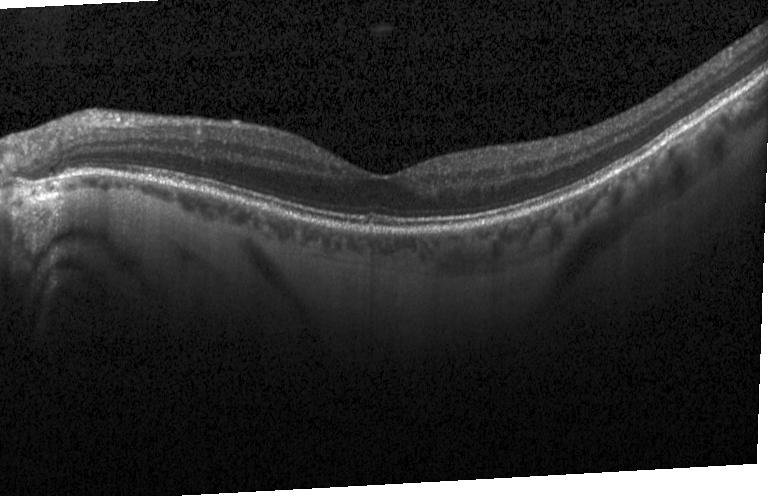 Dx: no choroidal neovascularization, no diabetic macular edema, and no drusen.